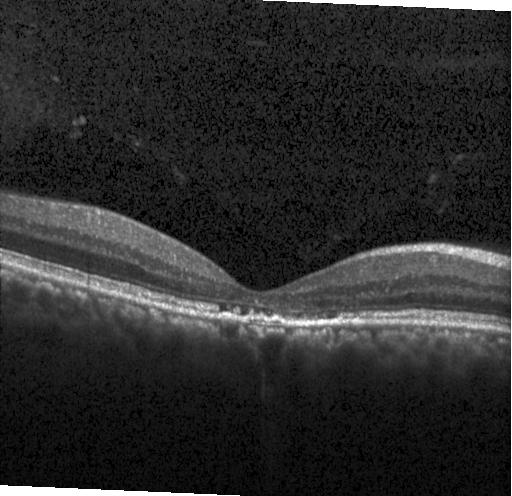

Spectral-domain OCT · acquired on a Heidelberg Spectralis · optical coherence tomography scan.
Macular OCT: choroidal neovascularization (CNV).